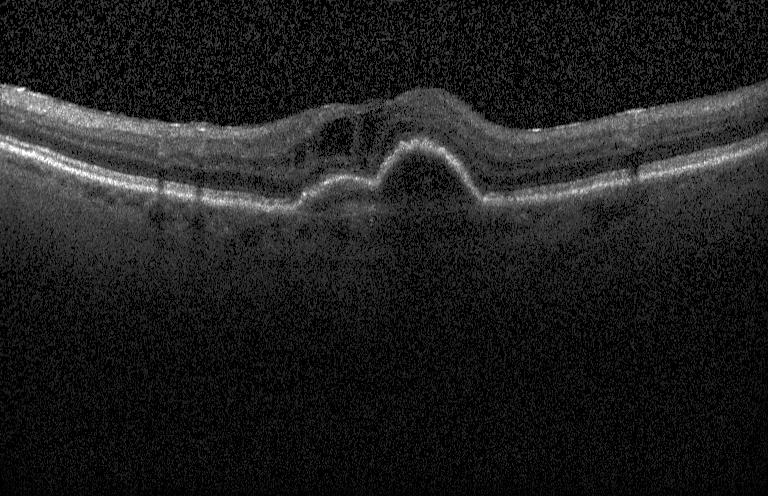
Retinal OCT B-scan, Heidelberg Spectralis OCT system, macular scan
The scan shows a choroidal neovascular membrane.